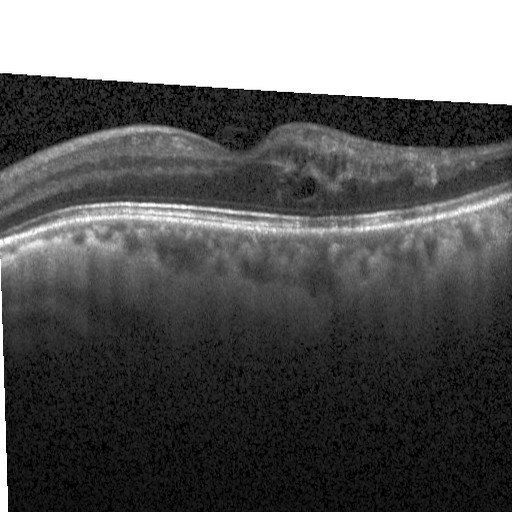 Retinal OCT cross-section showing DME.